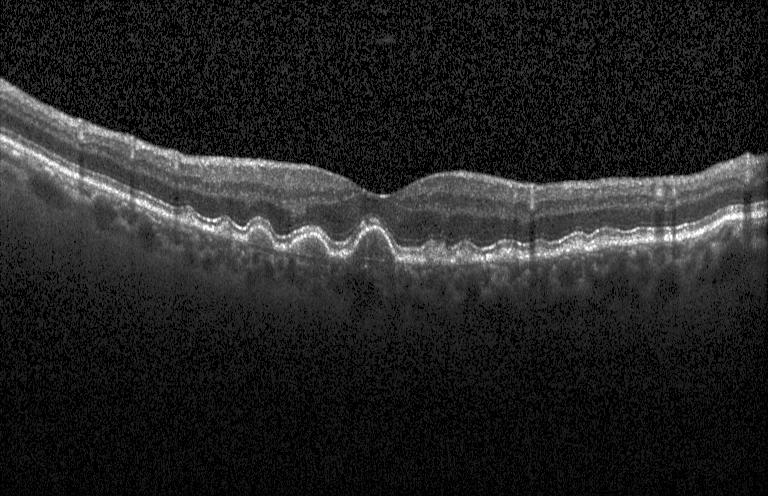 OCT B-scan, instrument: Heidelberg Spectralis.
Impression: drusen.